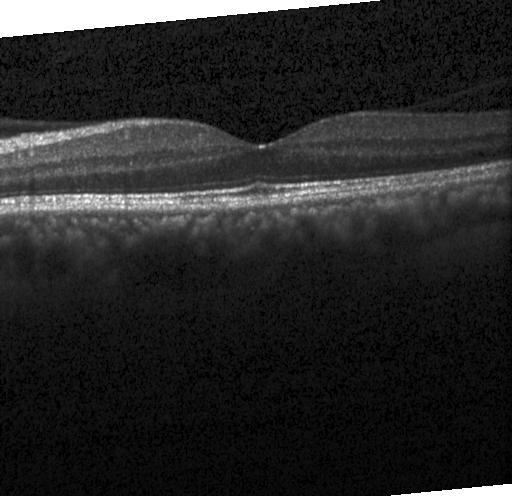

Centered on the fovea, optical coherence tomography scan.
Diagnosis: no choroidal neovascularization, no diabetic macular edema, and no drusen.